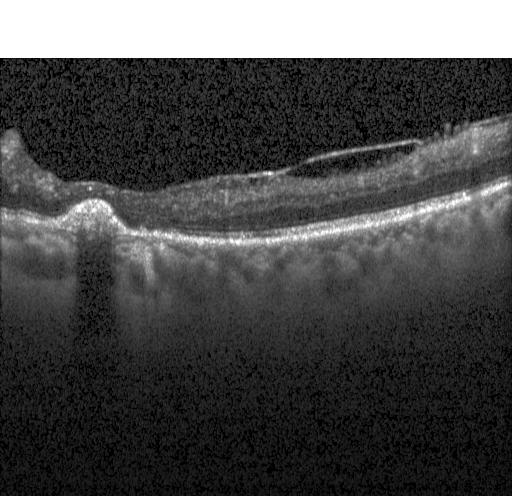

Instrument: Heidelberg Spectralis; retinal OCT cross-section
Impression: a choroidal neovascular membrane.